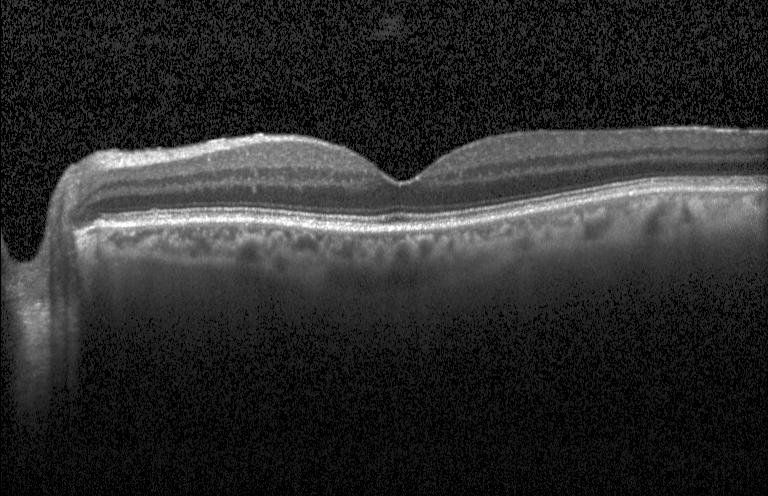 Instrument: Heidelberg Spectralis; spectral-domain optical coherence tomography; retinal OCT cross-section — Finding: no choroidal neovascularization, diabetic macular edema, or drusen.